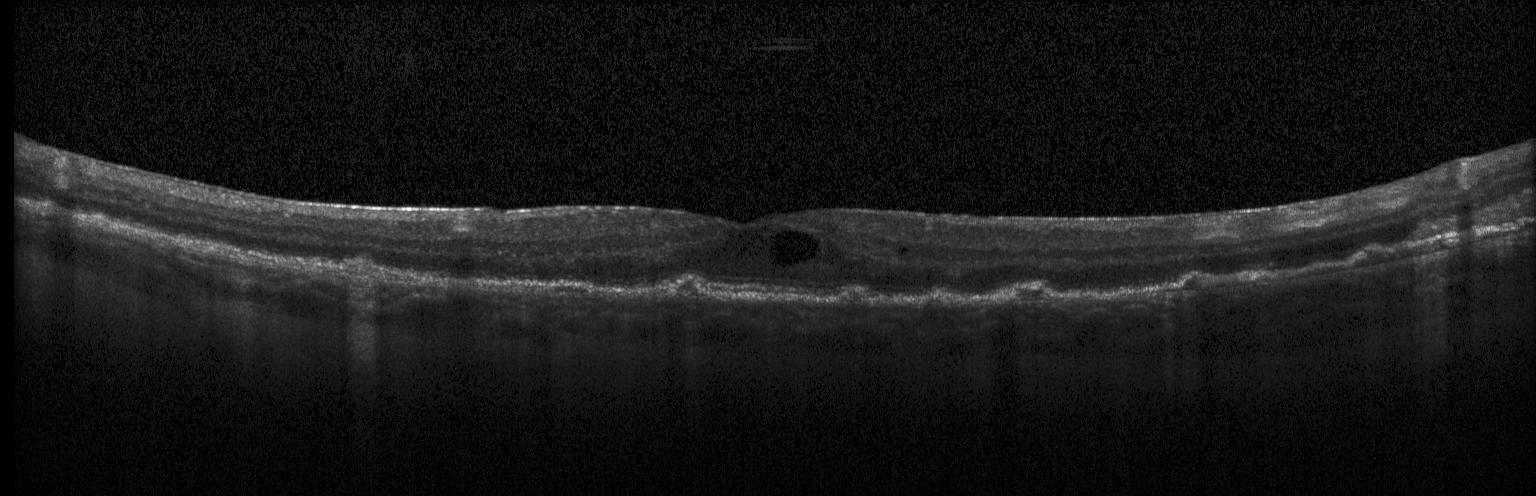
OCT line scan · horizontal scan through the fovea · spectral-domain OCT
Assessment: a choroidal neovascular membrane.